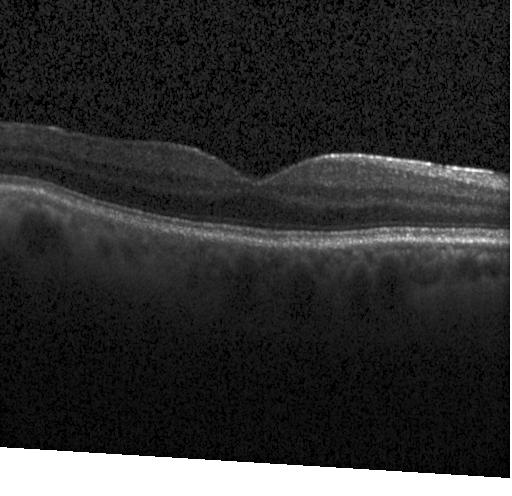 Spectral-domain OCT B-scan: neither choroidal neovascularization, diabetic macular edema, nor drusen.